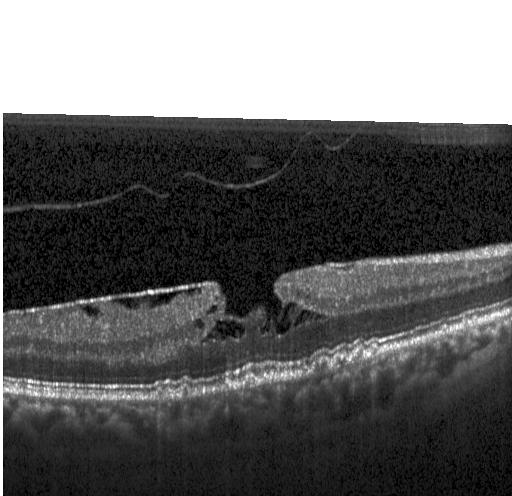

Finding: multiple drusen.